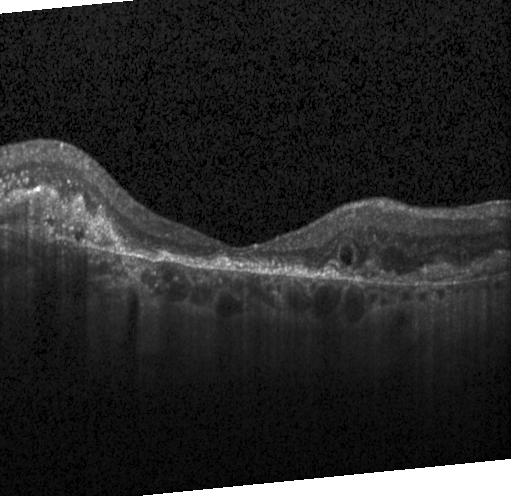

Impression: choroidal neovascularization.